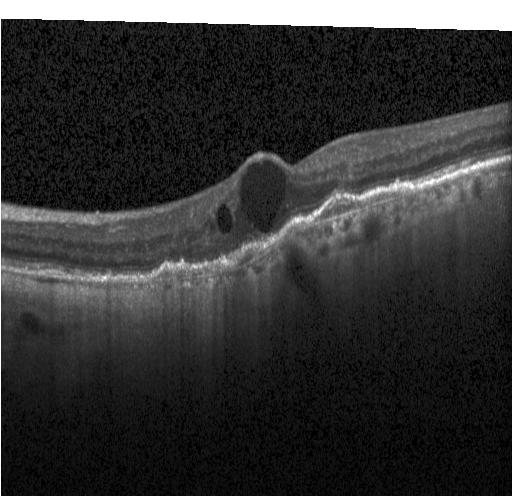
Finding: choroidal neovascularization.